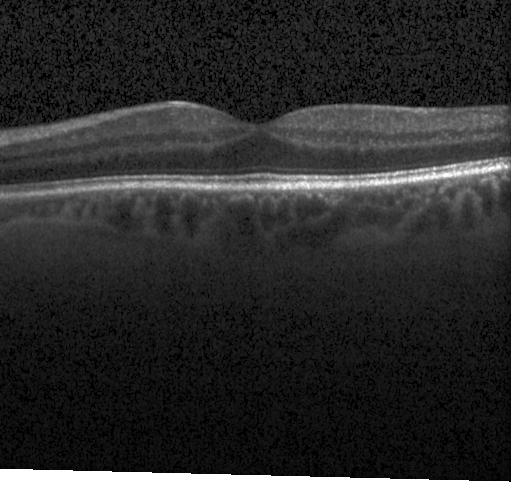
Finding: no evidence of choroidal neovascularization, diabetic macular edema, or drusen.